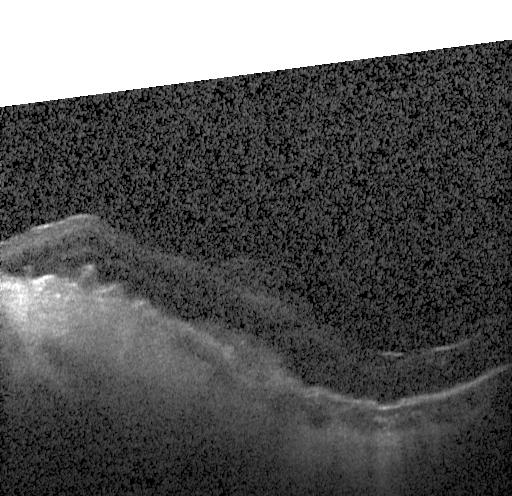
OCT finding: a choroidal neovascular membrane.